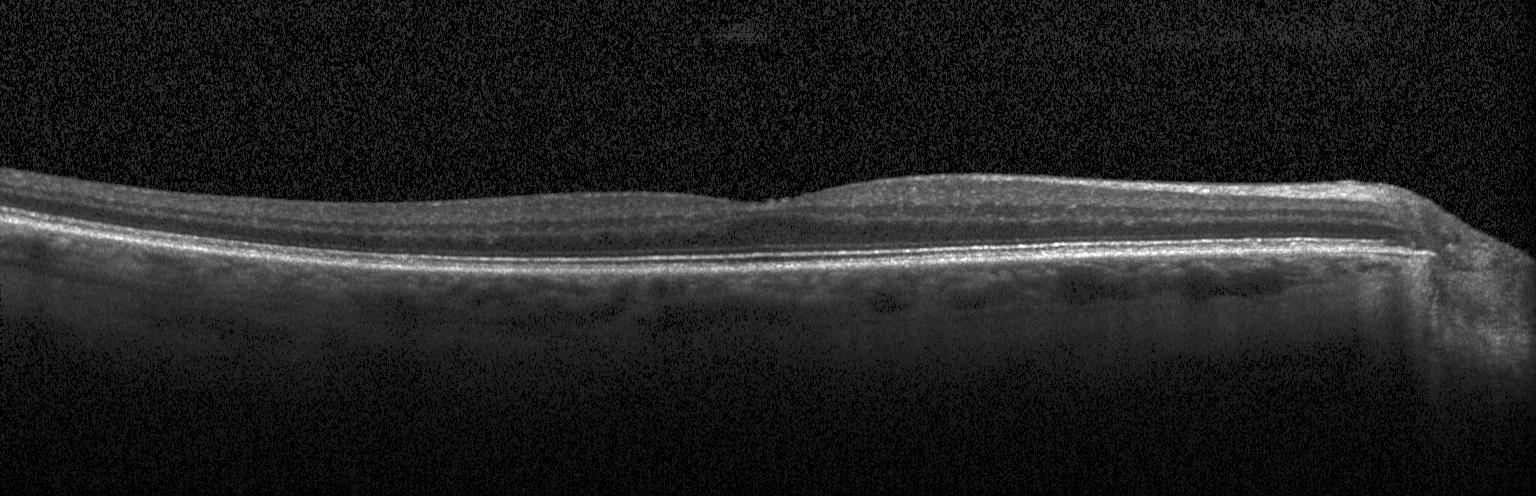 Assessment: no evidence of CNV, DME, or drusen.